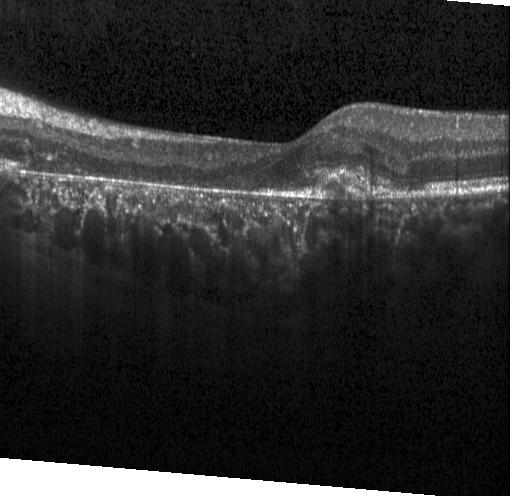

Retinal OCT cross-section — CNV.